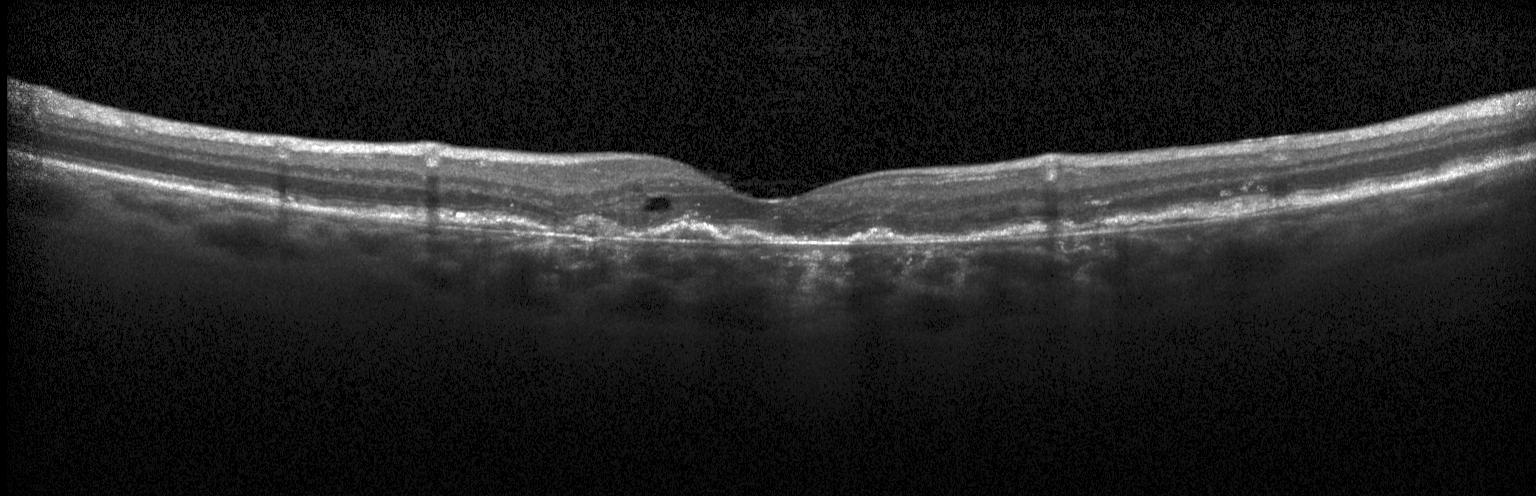
CNV.